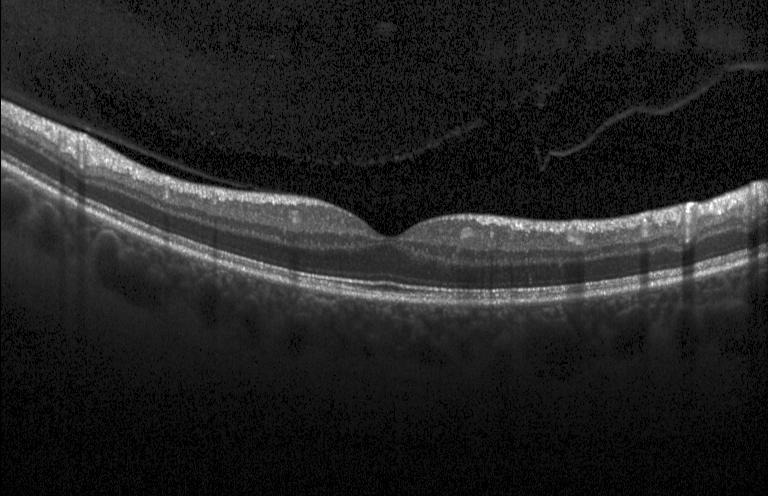 Retinal OCT B-scan.
The scan shows neither CNV, DME, nor drusen.